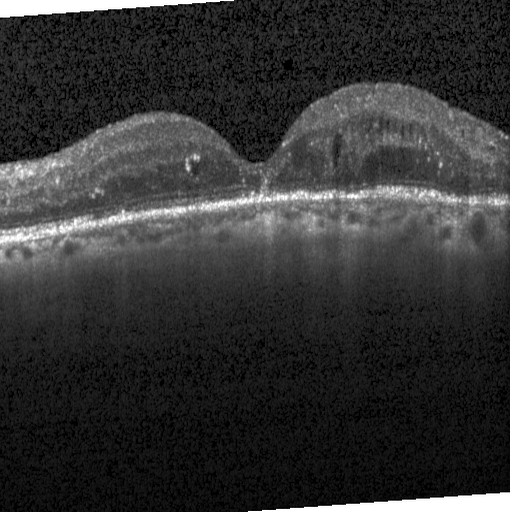

Fovea-centered · optical coherence tomography B-scan · SD-OCT.
Finding: diabetic macular edema (DME).